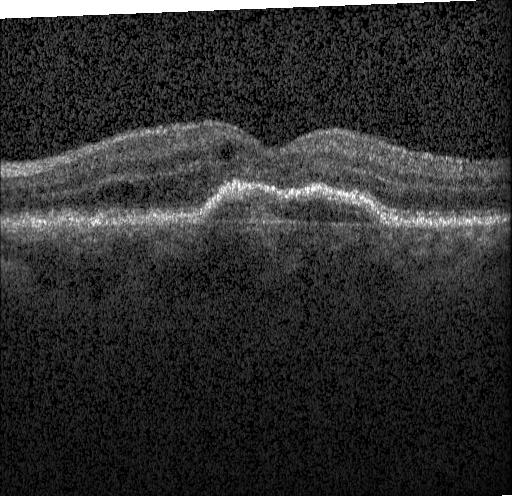

SD-OCT. Instrument: Heidelberg Spectralis. Macular scan. OCT B-scan. This B-scan demonstrates a choroidal neovascular membrane.